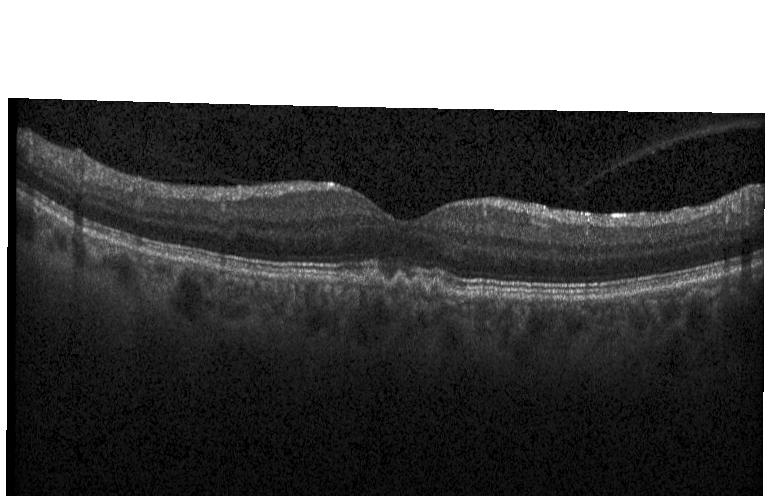 Optical coherence tomography B-scan.
Impression: drusen.